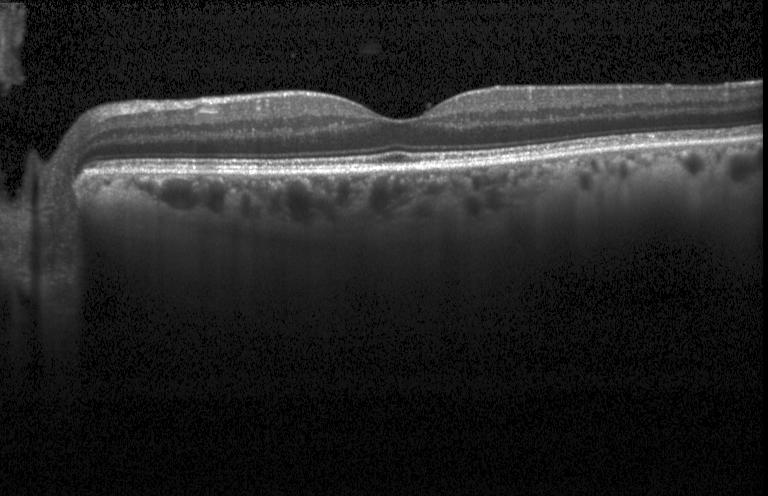
Acquired on a Heidelberg Spectralis, SD-OCT, retinal OCT cross-section, through the macula.
OCT finding: neither choroidal neovascularization, diabetic macular edema, nor drusen.